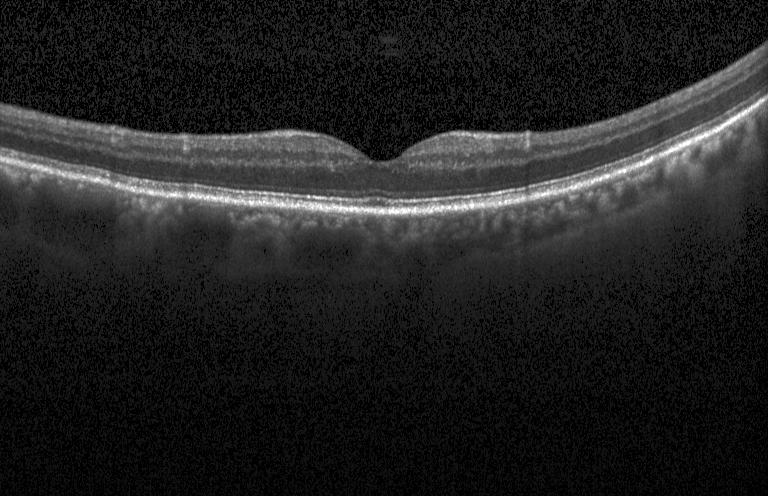
Optical coherence tomography B-scan; acquired on a Heidelberg Spectralis; spectral-domain OCT — Diagnosis: neither CNV, DME, nor drusen.